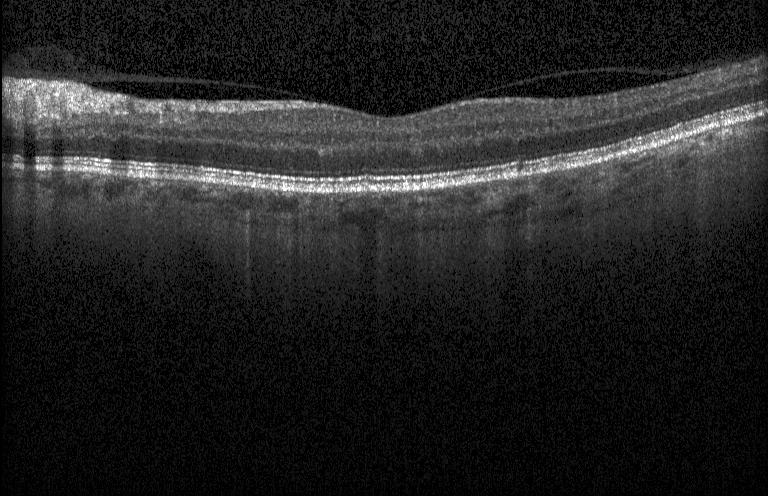 The scan shows no evidence of choroidal neovascularization, diabetic macular edema, or drusen.